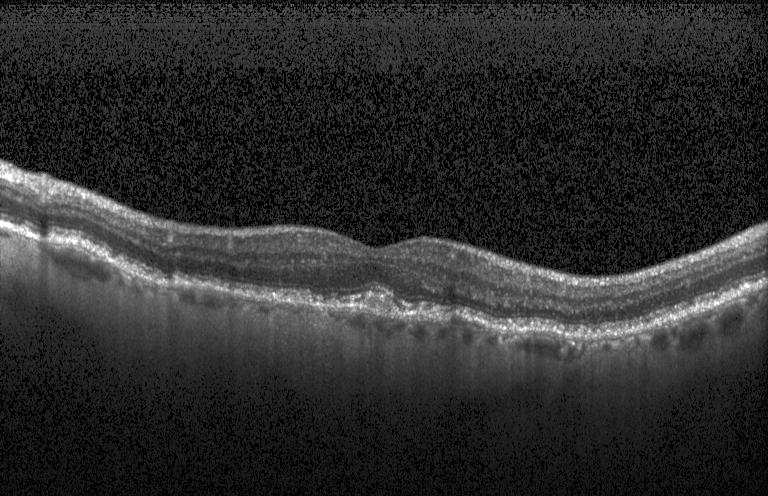

Macular OCT: drusen.